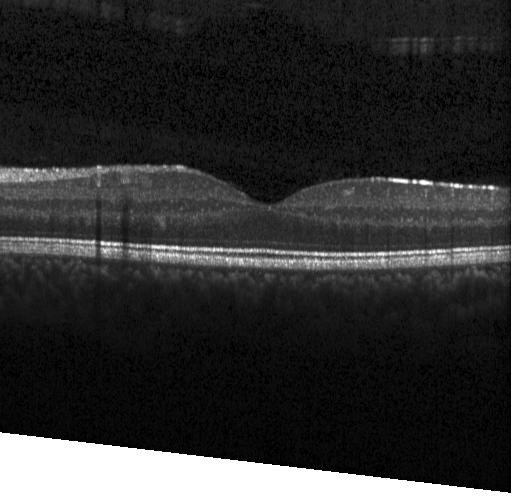
The scan shows no CNV, no DME, and no drusen.